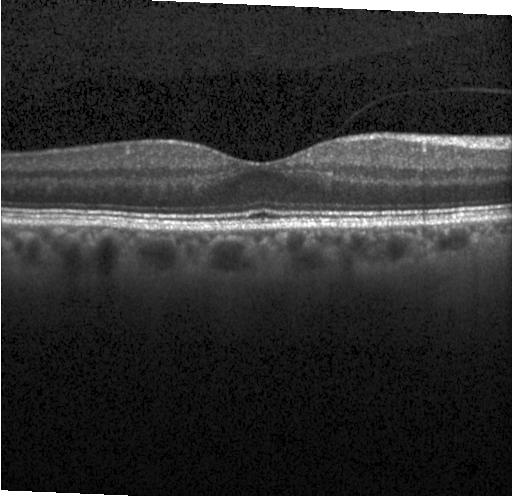 Dx: no choroidal neovascularization, diabetic macular edema, or drusen.